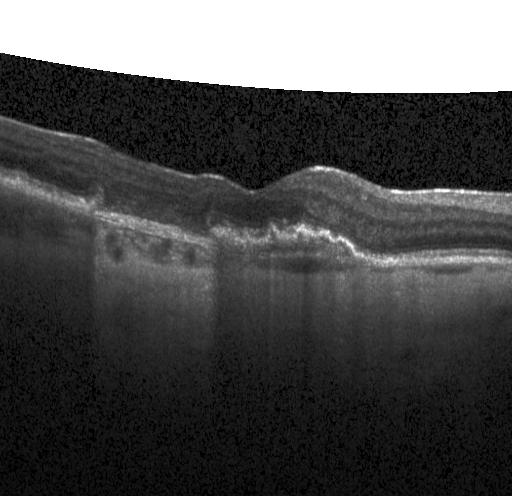

Macular scan · retinal OCT cross-section · acquired on a Heidelberg Spectralis · spectral-domain OCT.
Dx: a choroidal neovascular membrane.